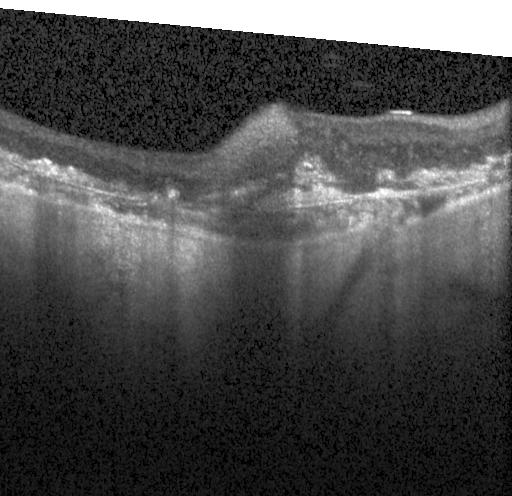

Diagnosis: a choroidal neovascular membrane.